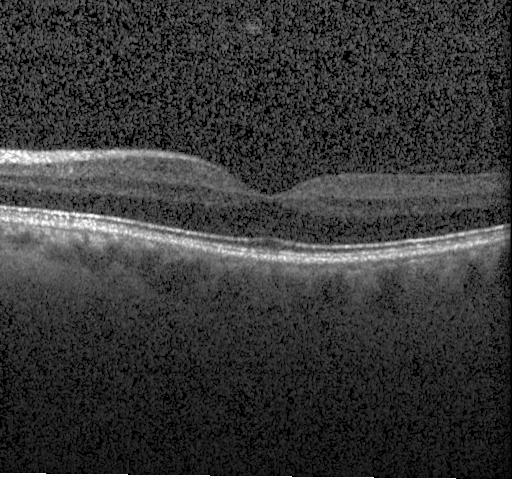 This B-scan demonstrates neither choroidal neovascularization, diabetic macular edema, nor drusen.